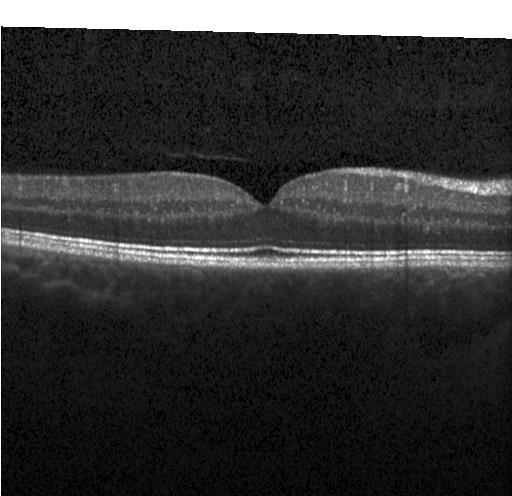

Heidelberg Spectralis OCT system, OCT B-scan, macular scan, SD-OCT.
Impression: neither choroidal neovascularization, diabetic macular edema, nor drusen.